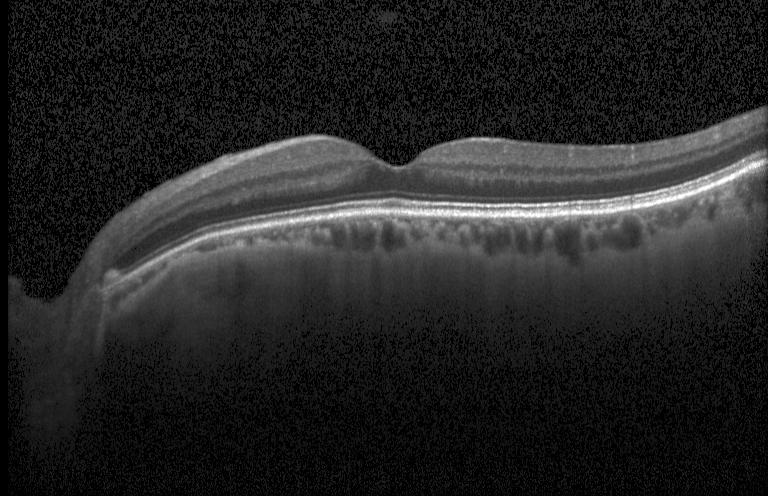

Optical coherence tomography B-scan; instrument: Heidelberg Spectralis. Finding: no evidence of choroidal neovascularization, diabetic macular edema, or drusen.